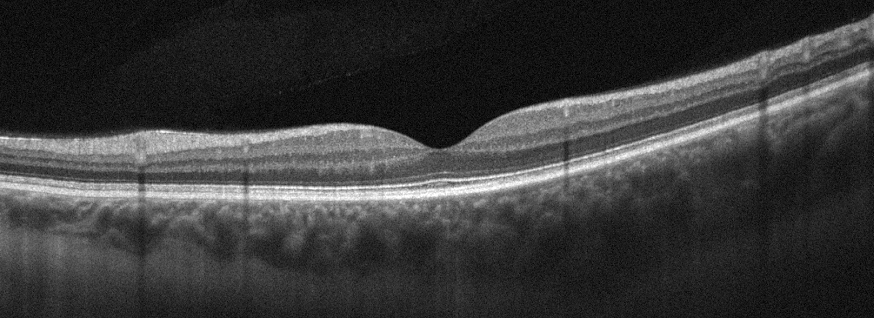
Assessment: absence of AMD, DME, ERM, RAO, RVO, and vitreomacular interface disease.